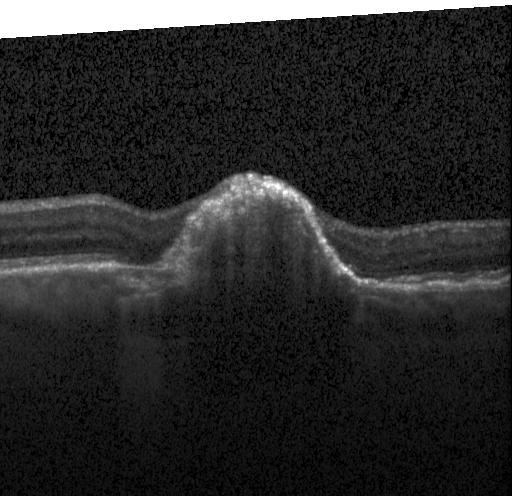

Dx: choroidal neovascularization (CNV).